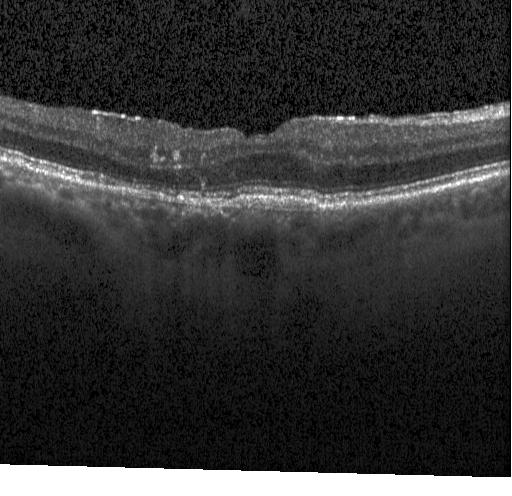 Centered on the fovea · spectral-domain OCT · OCT line scan.
Diagnosis: a choroidal neovascular membrane.